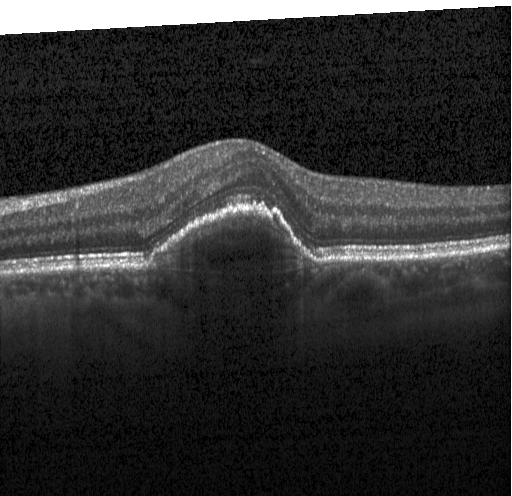
OCT B-scan; acquired on a Heidelberg Spectralis; macular scan — Assessment: choroidal neovascularization.